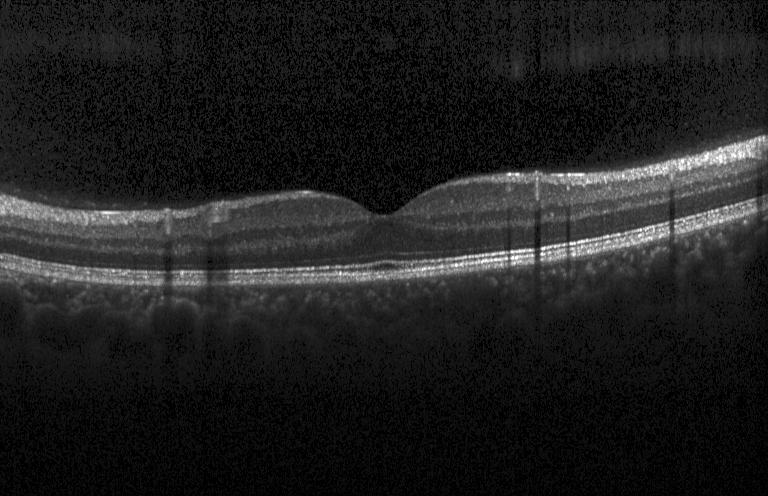 Spectral-domain OCT. Retinal OCT cross-section. Heidelberg Spectralis OCT system. Macular scan — No evidence of choroidal neovascularization, diabetic macular edema, or drusen.